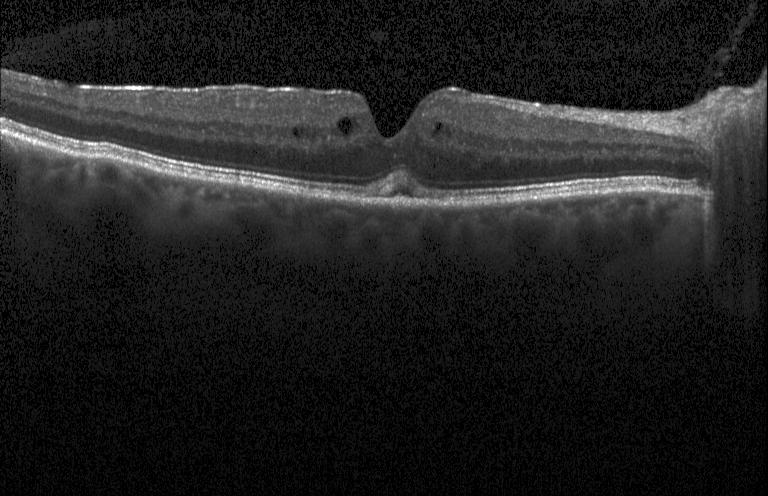

Spectral-domain OCT; optical coherence tomography B-scan; acquired on a Heidelberg Spectralis. This B-scan demonstrates diabetic macular edema (DME).